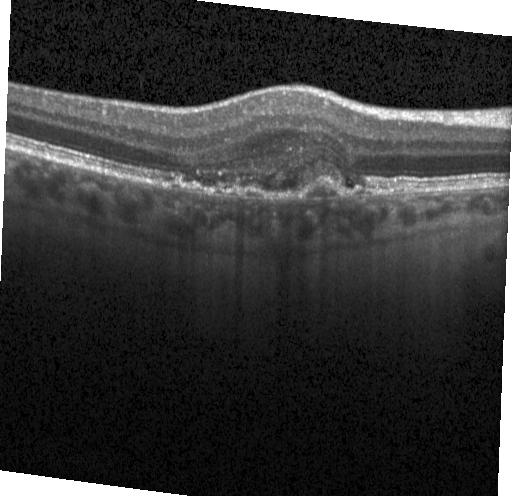
Retinal OCT cross-section showing choroidal neovascularization (CNV).